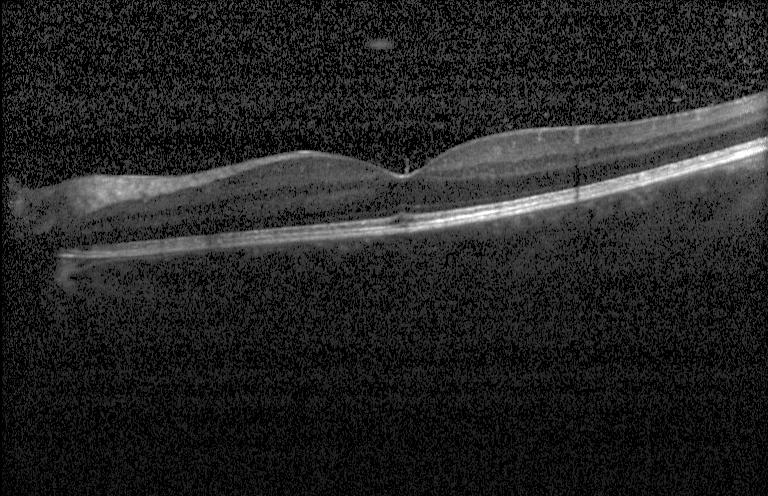 Spectral-domain optical coherence tomography; retinal OCT cross-section. The scan shows neither choroidal neovascularization, diabetic macular edema, nor drusen.